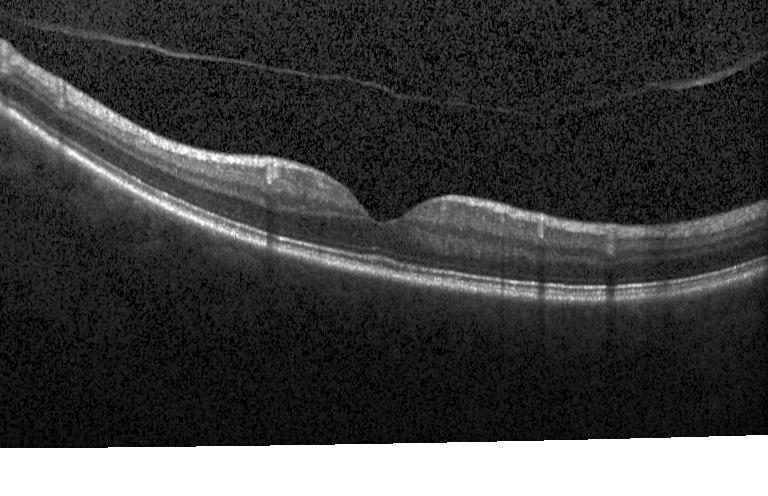 Retinal OCT cross-section showing neither CNV, DME, nor drusen.